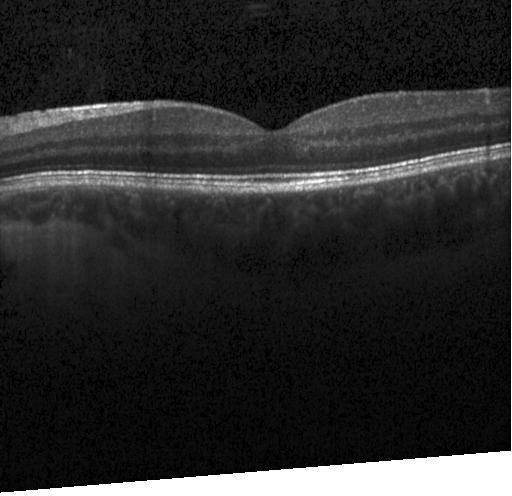 Retinal OCT B-scan. Fovea-centered. Spectral-domain optical coherence tomography
The scan shows no choroidal neovascularization, diabetic macular edema, or drusen.